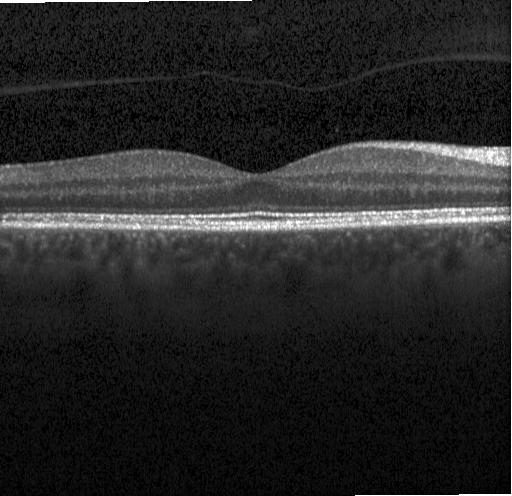

Through the macula, optical coherence tomography scan, SD-OCT, acquired on a Heidelberg Spectralis
Impression: no CNV, no DME, and no drusen.